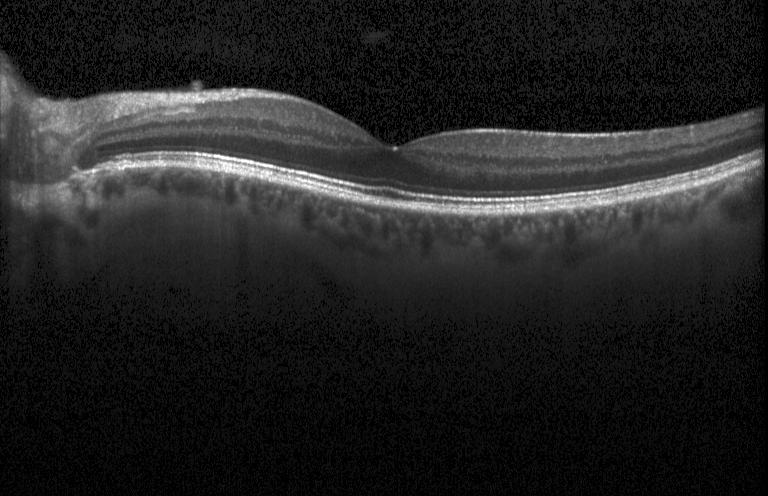

Macular OCT demonstrating no choroidal neovascularization, diabetic macular edema, or drusen.